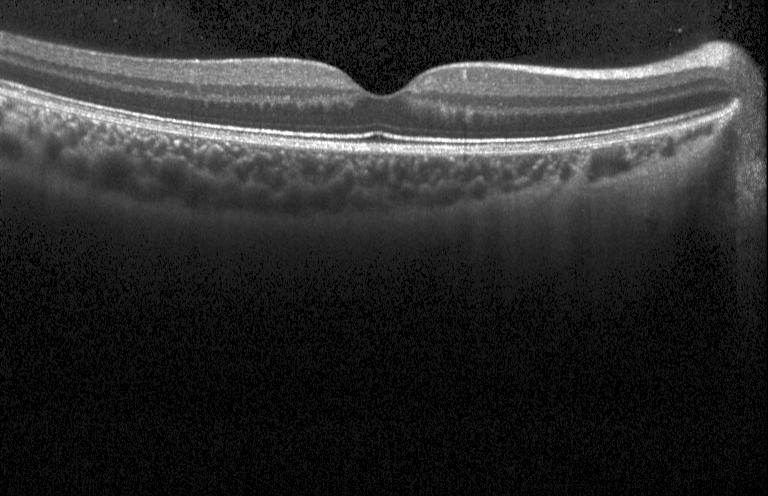 Optical coherence tomography scan. Horizontal scan through the fovea. OCT finding: no choroidal neovascularization, no diabetic macular edema, and no drusen.